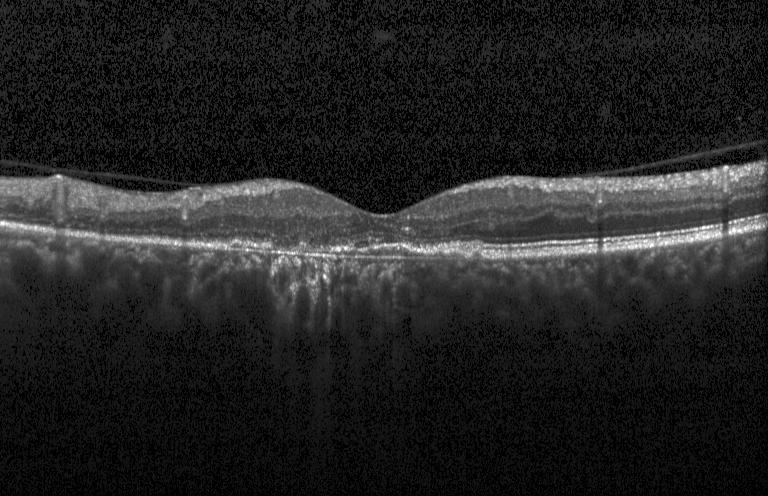

The scan shows choroidal neovascularization (CNV).